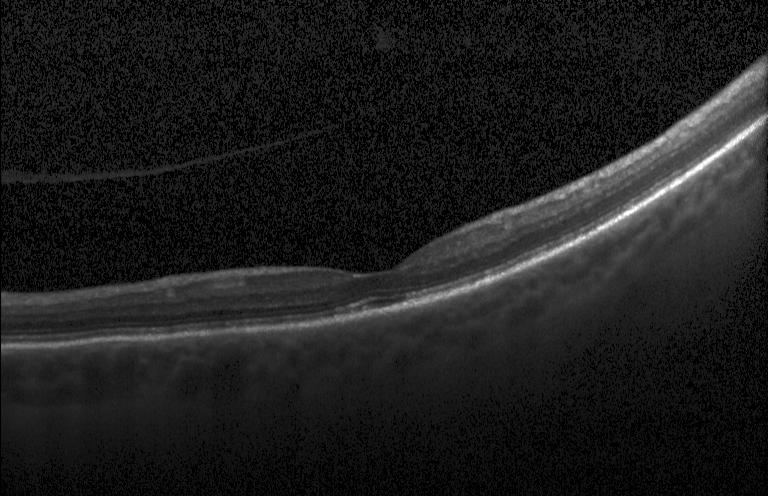 OCT line scan.
Macular OCT: no evidence of CNV, DME, or drusen.